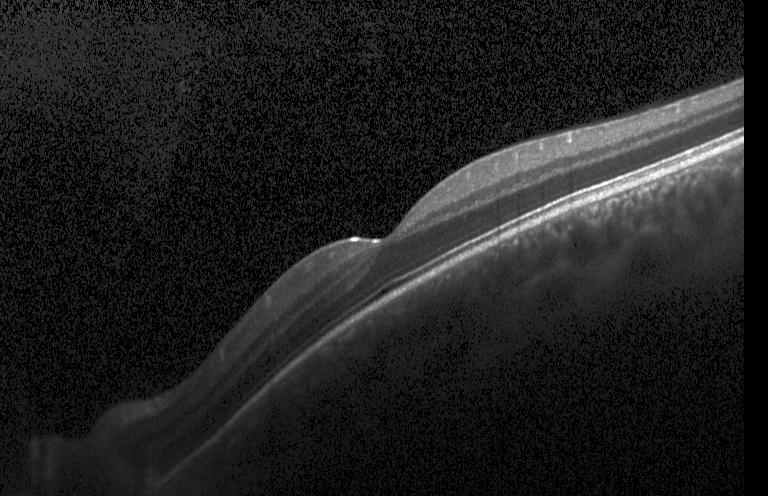

Retinal OCT B-scan.
Dx: no CNV, no DME, and no drusen.